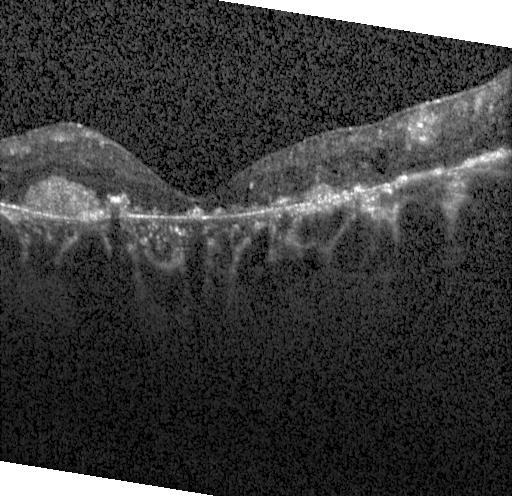
Heidelberg Spectralis OCT system, OCT line scan. Finding: a choroidal neovascular membrane.